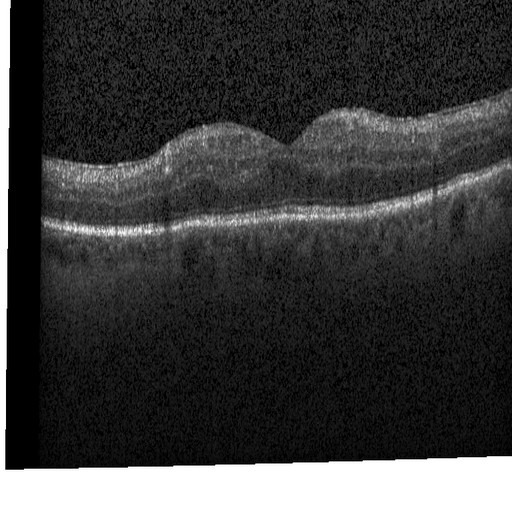
Spectral-domain OCT; retinal OCT cross-section; acquired on a Heidelberg Spectralis.
Assessment: DME.